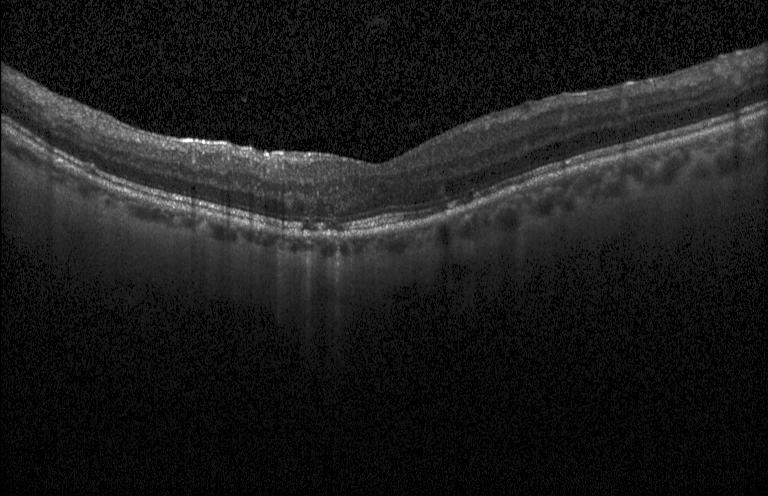

The scan shows no evidence of choroidal neovascularization, diabetic macular edema, or drusen.